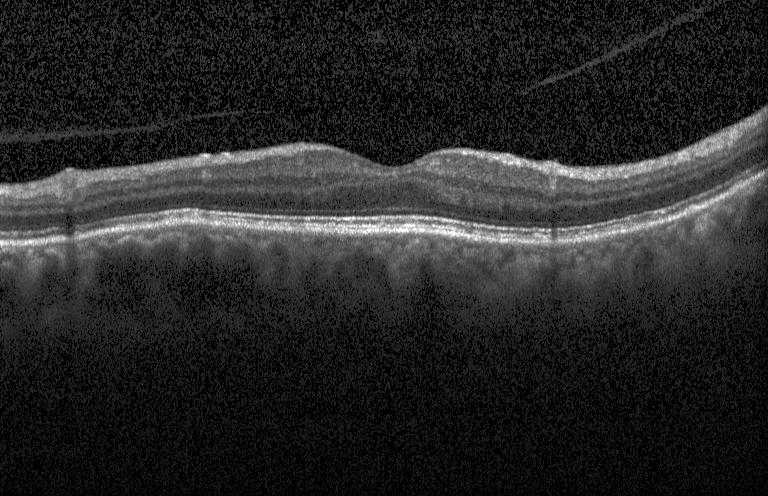

Retinal OCT cross-section.
Dx: neither choroidal neovascularization, diabetic macular edema, nor drusen.